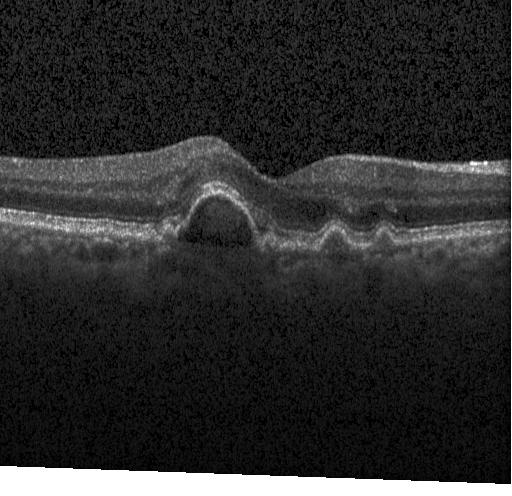

Spectral-domain optical coherence tomography; OCT line scan — Dx: a choroidal neovascular membrane.